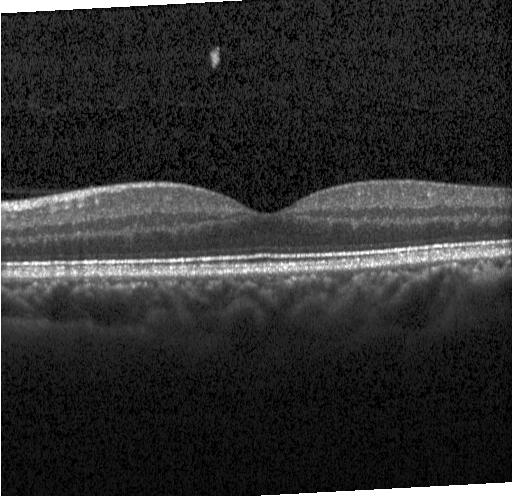
SD-OCT; Heidelberg Spectralis OCT system; optical coherence tomography B-scan; through the macula. Impression: no CNV, no DME, and no drusen.